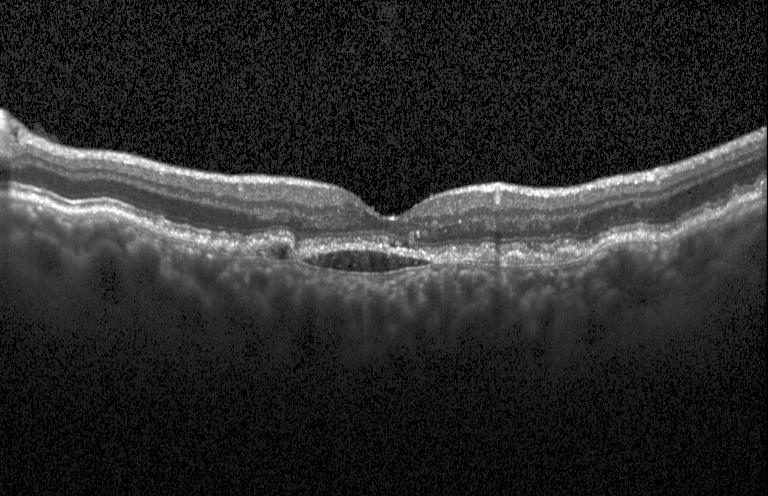

The scan shows choroidal neovascularization.